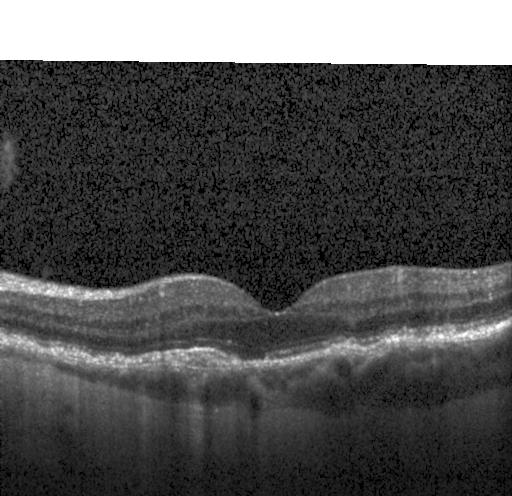

Dx: CNV.